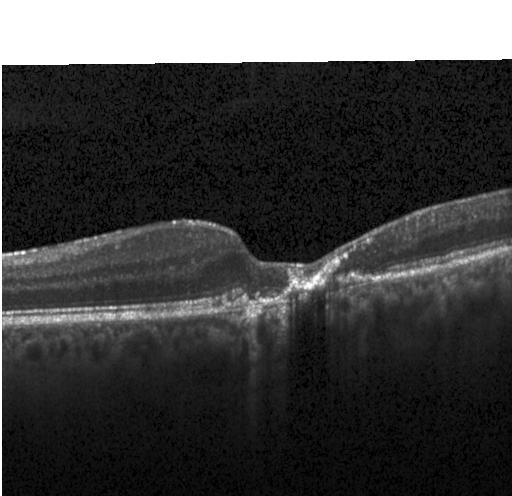
Optical coherence tomography scan, horizontal scan through the fovea.
OCT finding: a choroidal neovascular membrane.